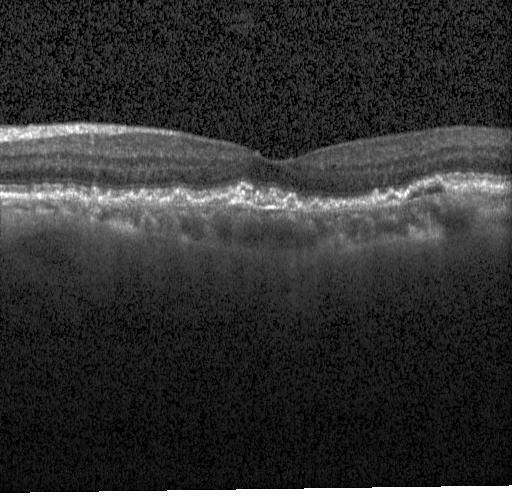
Optical coherence tomography B-scan.
Diagnosis: drusen.